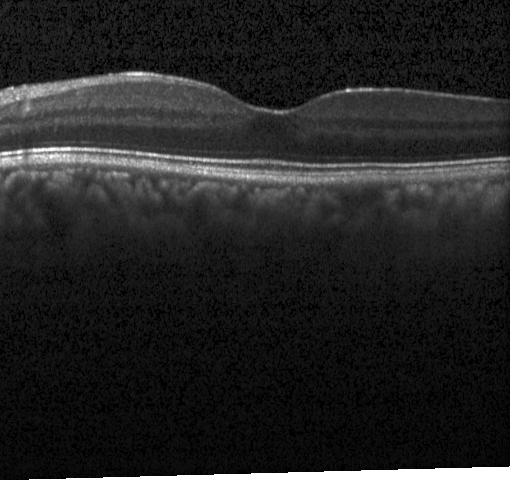
Finding: no CNV, DME, or drusen.